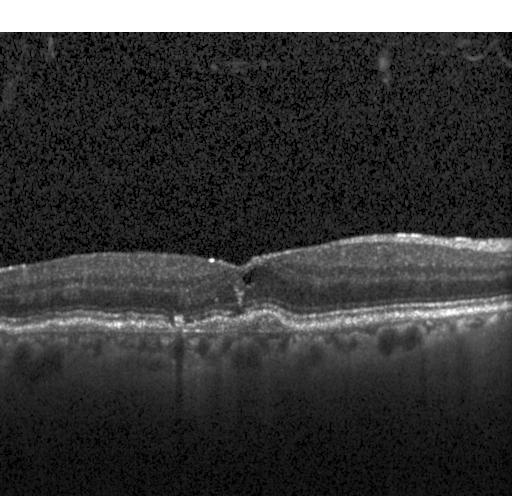
The scan shows a choroidal neovascular membrane.